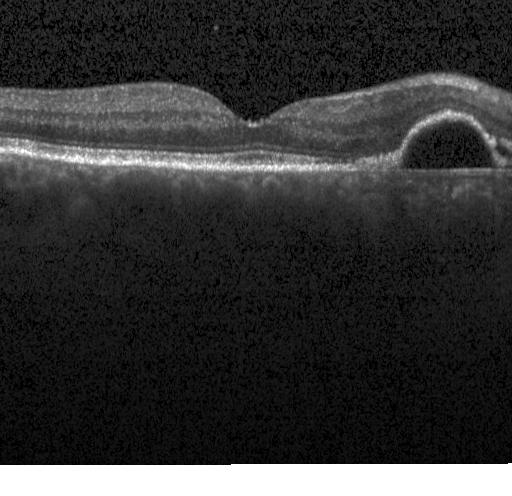
Optical coherence tomography B-scan; Heidelberg Spectralis OCT system; spectral-domain OCT; centered on the fovea. Dx: a choroidal neovascular membrane.